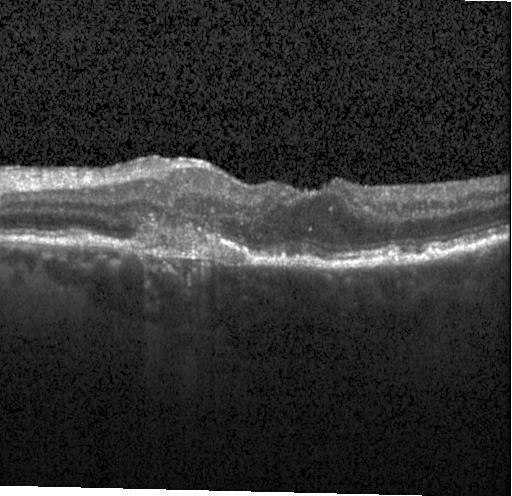

SD-OCT · OCT line scan · acquired on a Heidelberg Spectralis · through the macula
Dx: choroidal neovascularization (CNV).